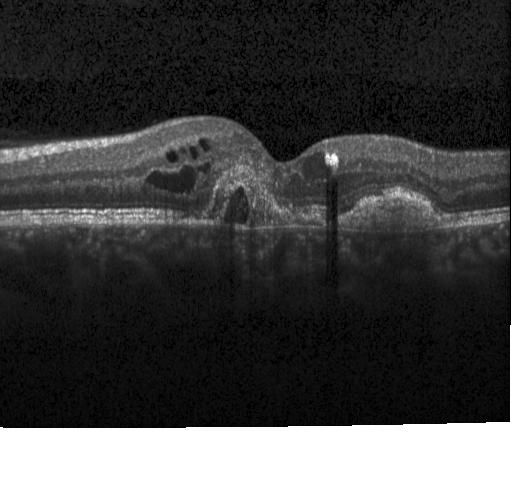 Heidelberg Spectralis · spectral-domain optical coherence tomography · horizontal scan through the fovea · retinal OCT B-scan
This B-scan demonstrates choroidal neovascularization (CNV).